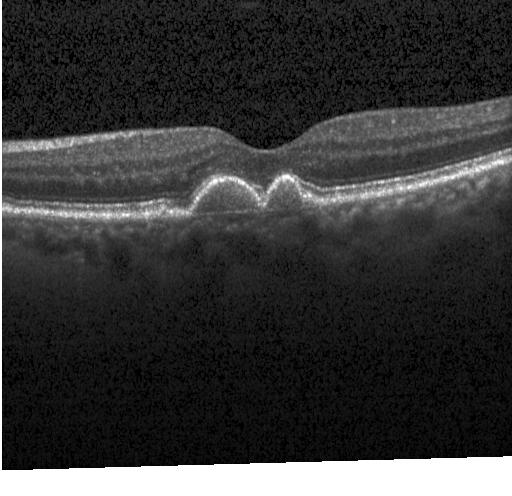

Optical coherence tomography B-scan
OCT finding: sub-RPE drusenoid deposits.